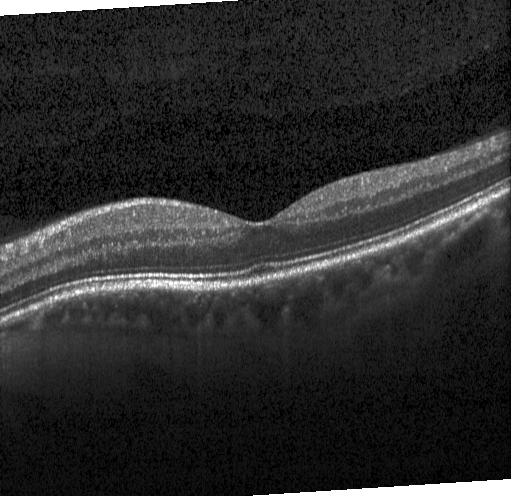 Fovea-centered · OCT B-scan · SD-OCT
Impression: no evidence of CNV, DME, or drusen.